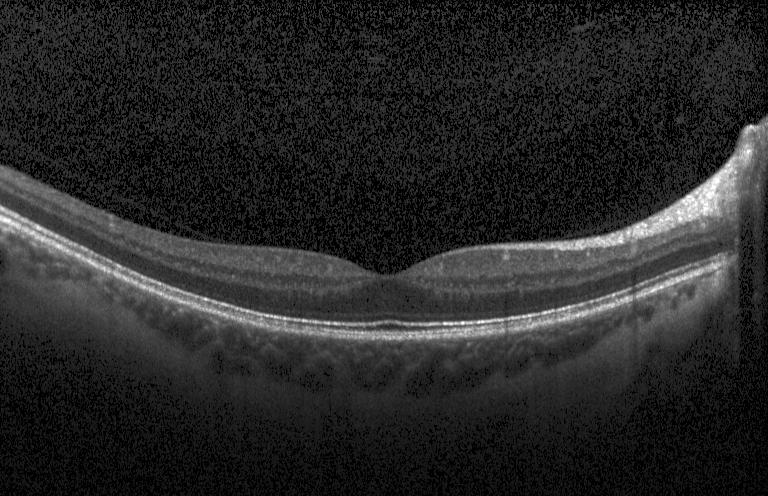 Macular OCT demonstrating no CNV, no DME, and no drusen.